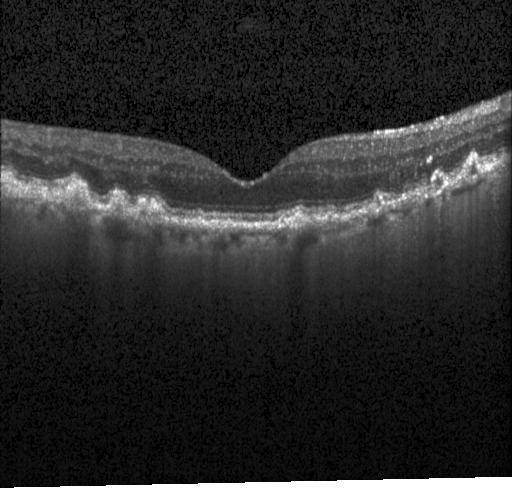

Optical coherence tomography B-scan, centered on the fovea, spectral-domain optical coherence tomography
Finding: drusen.